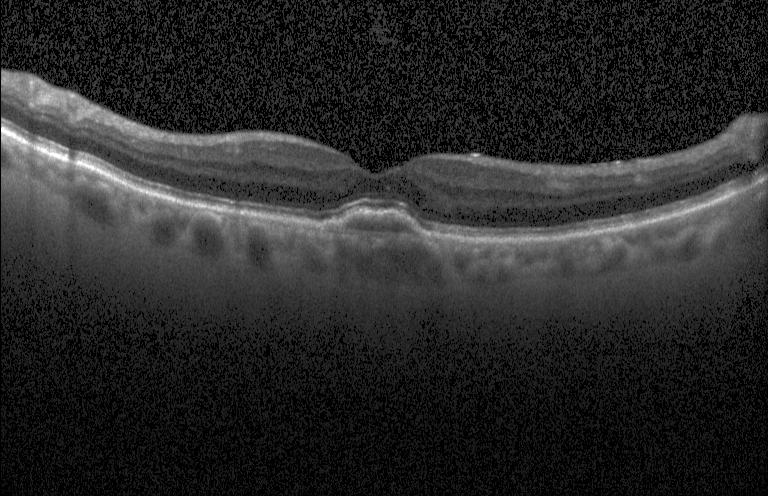 SD-OCT · macular scan · instrument: Heidelberg Spectralis · OCT line scan. Diagnosis: choroidal neovascularization (CNV).